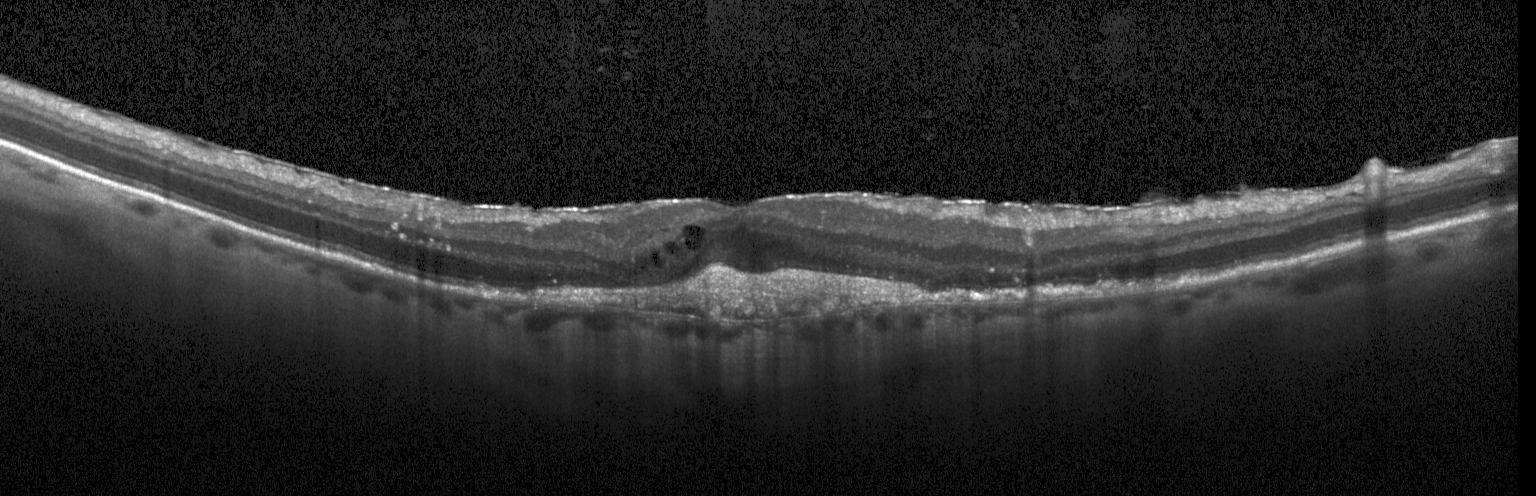

OCT B-scan showing a choroidal neovascular membrane.